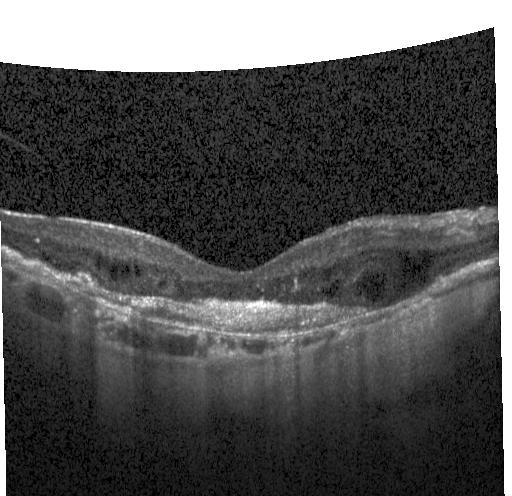 OCT B-scan; Heidelberg Spectralis; macular scan; SD-OCT — Dx: CNV.